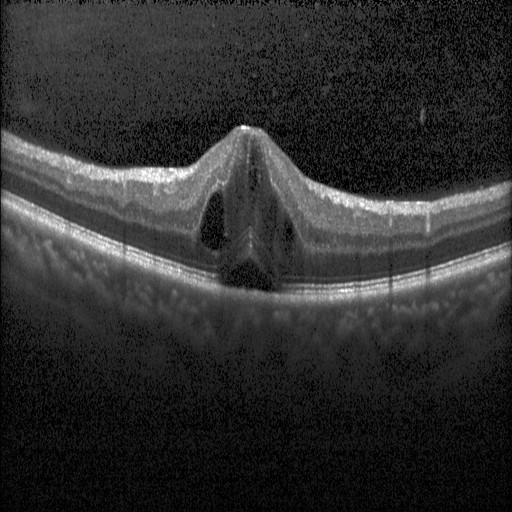

Optical coherence tomography scan — Finding: diabetic macular edema (DME).